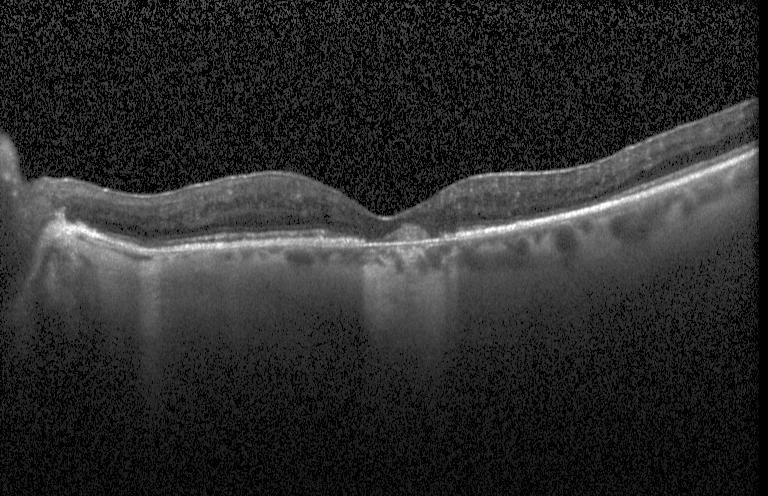 Spectral-domain optical coherence tomography · retinal OCT B-scan — The scan shows choroidal neovascularization (CNV).